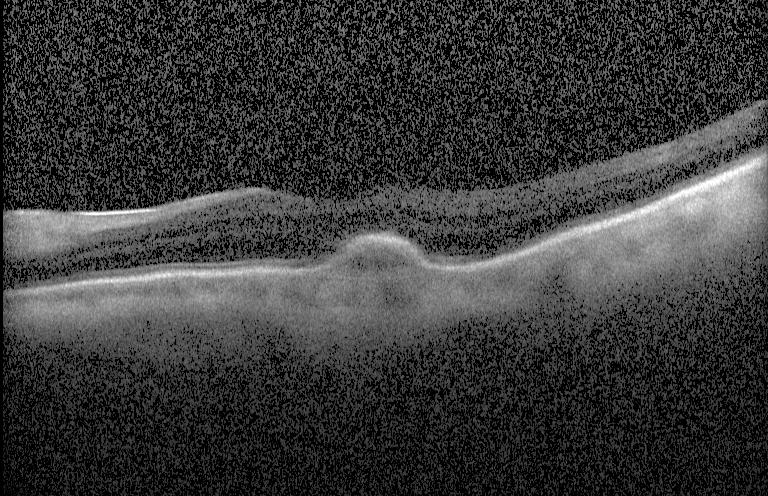
OCT B-scan
Finding: a choroidal neovascular membrane.